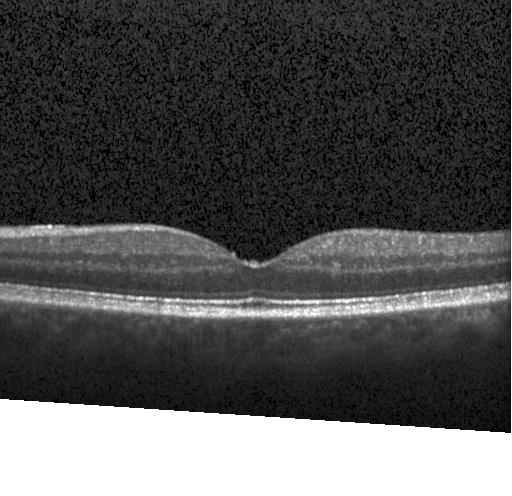

Horizontal scan through the fovea · optical coherence tomography scan
Neither CNV, DME, nor drusen.